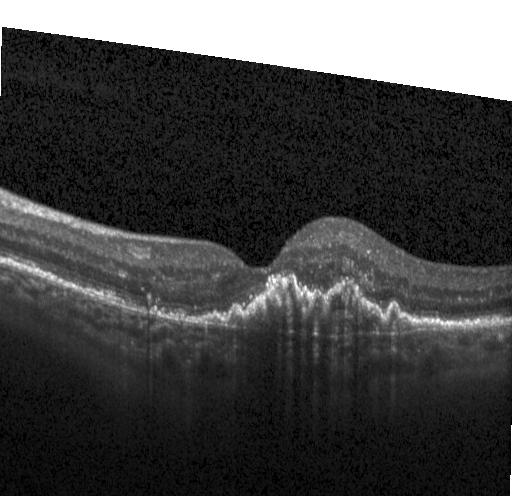 Finding: choroidal neovascularization.